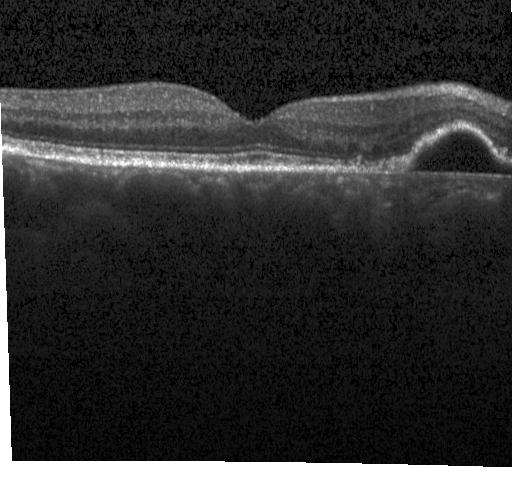

Spectral-domain optical coherence tomography. Optical coherence tomography B-scan
Finding: a choroidal neovascular membrane.